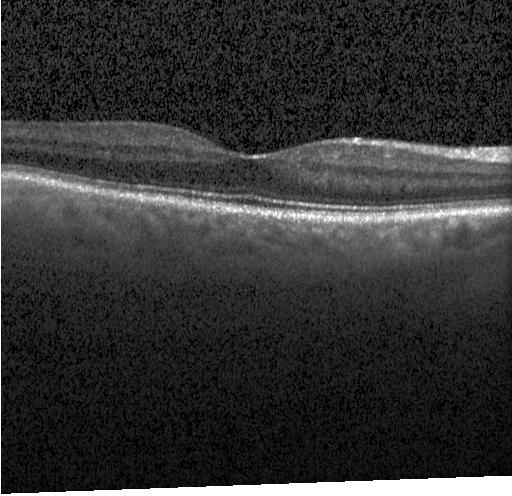
Horizontal scan through the fovea · retinal OCT B-scan · Heidelberg Spectralis OCT system · SD-OCT — Assessment: no evidence of choroidal neovascularization, diabetic macular edema, or drusen.